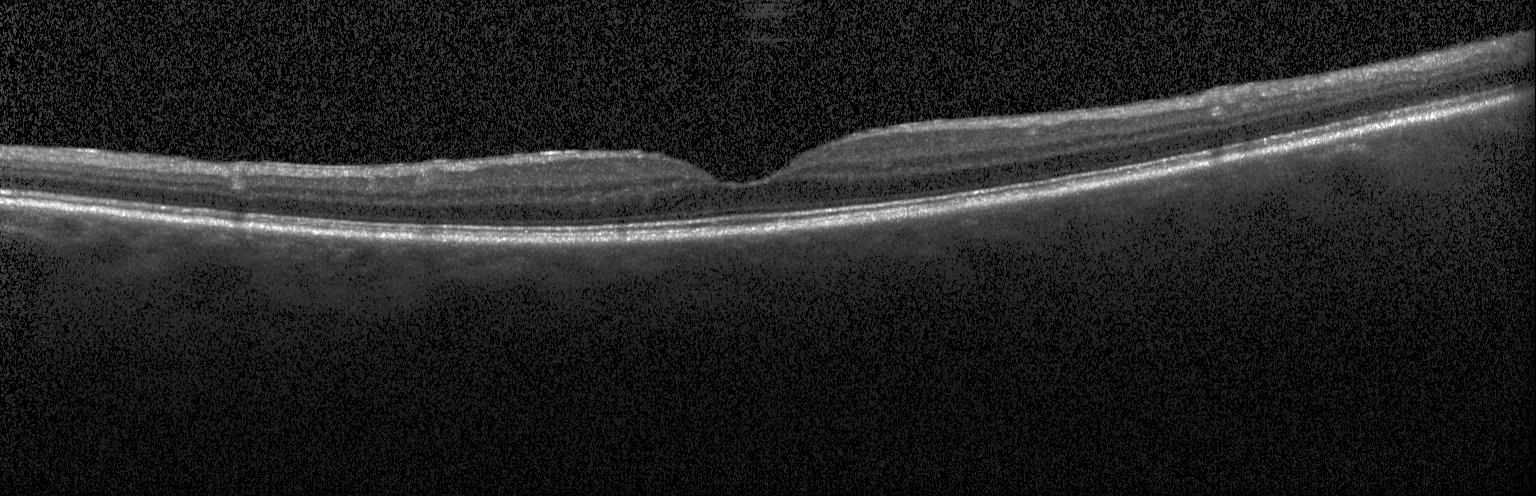 OCT line scan; acquired on a Heidelberg Spectralis. Diagnosis: no choroidal neovascularization, no diabetic macular edema, and no drusen.